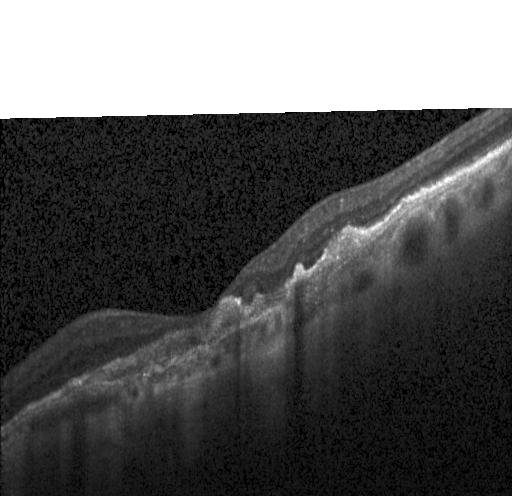
Acquired on a Heidelberg Spectralis. Spectral-domain OCT. Retinal OCT cross-section — Impression: CNV.